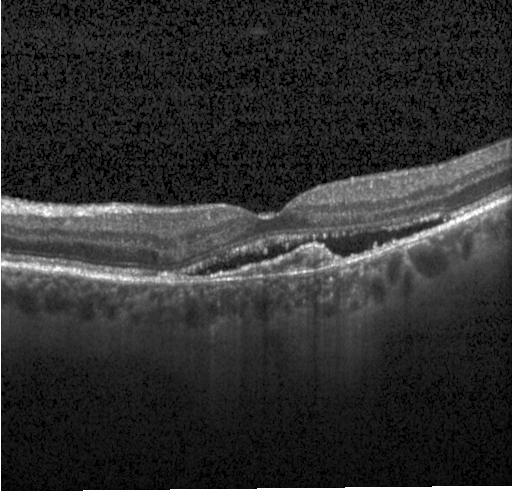
Through the macula, spectral-domain OCT, instrument: Heidelberg Spectralis, optical coherence tomography B-scan. Diagnosis: choroidal neovascularization.